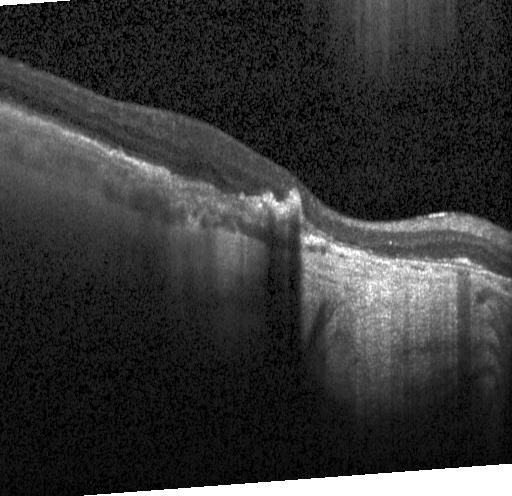 Diagnosis: choroidal neovascularization (CNV).